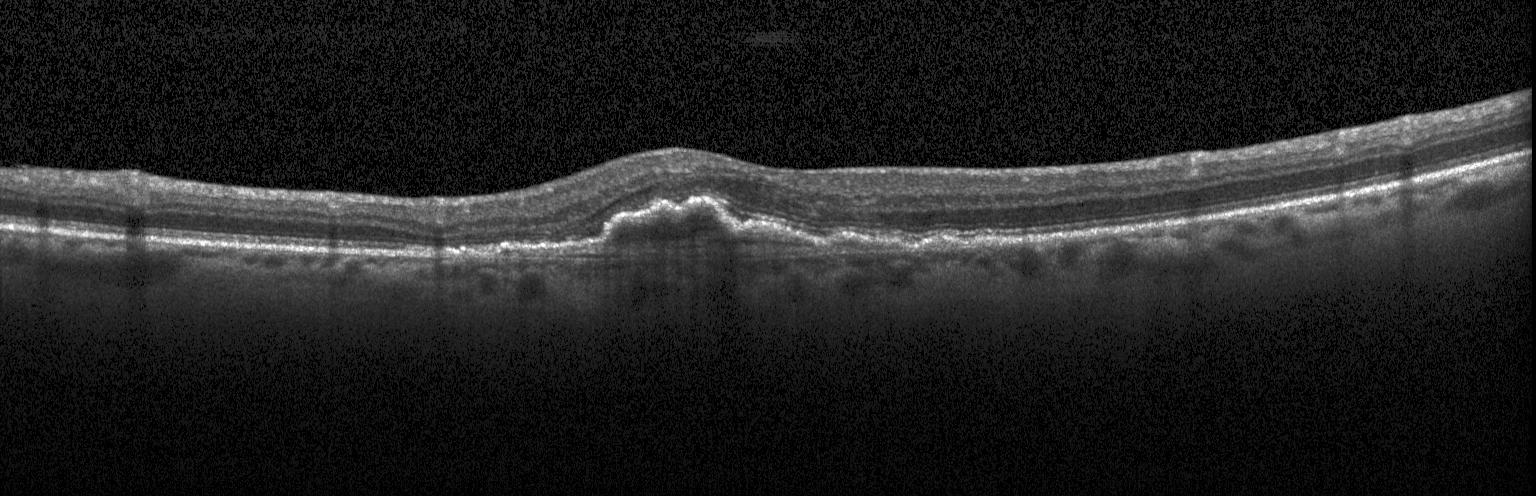 This B-scan demonstrates a choroidal neovascular membrane.